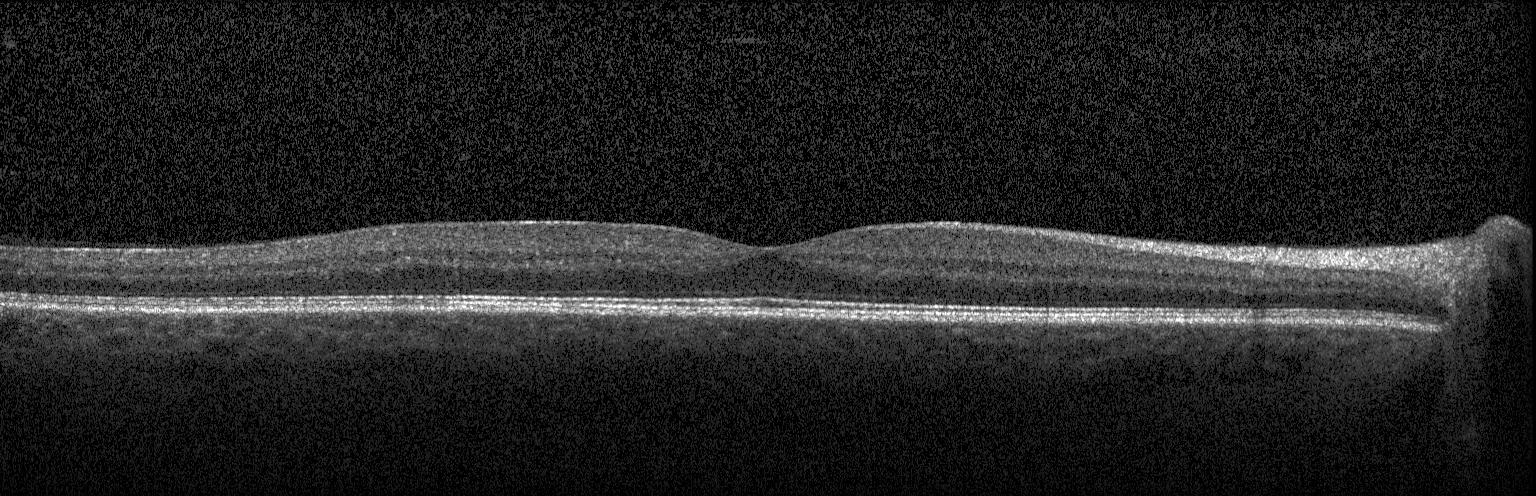

OCT scan showing neither choroidal neovascularization, diabetic macular edema, nor drusen.